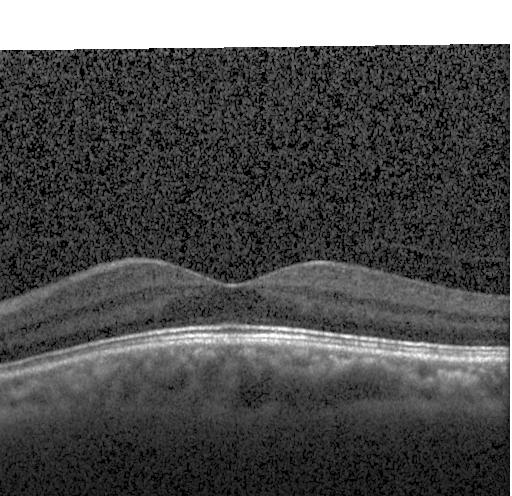
No CNV, DME, or drusen.